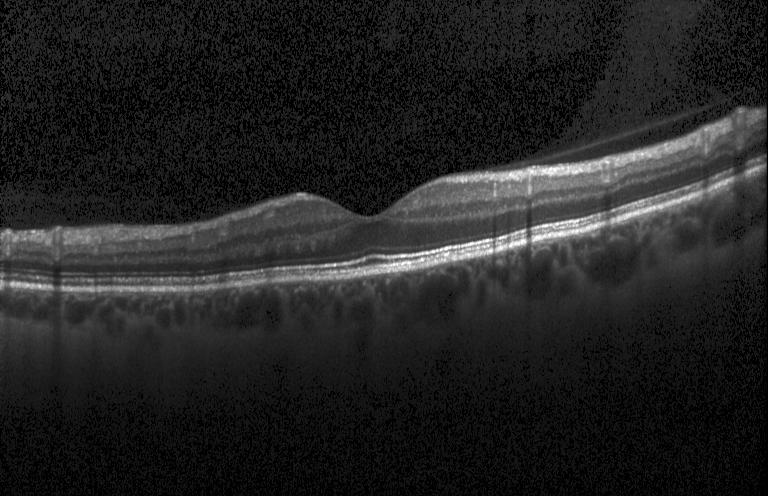

Macular scan; Heidelberg Spectralis; spectral-domain optical coherence tomography; retinal OCT B-scan. Diagnosis: neither choroidal neovascularization, diabetic macular edema, nor drusen.